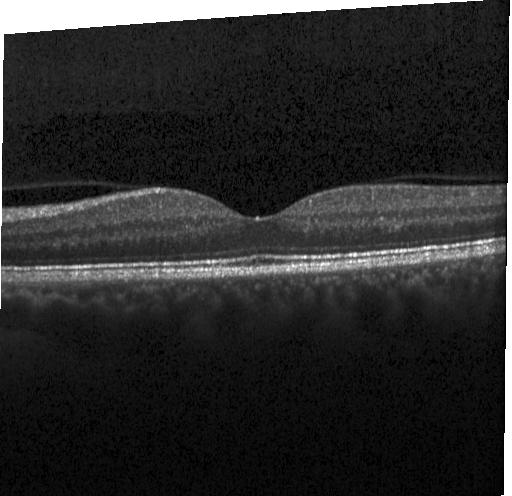 Centered on the fovea · instrument: Heidelberg Spectralis · optical coherence tomography B-scan. The scan shows no choroidal neovascularization, diabetic macular edema, or drusen.